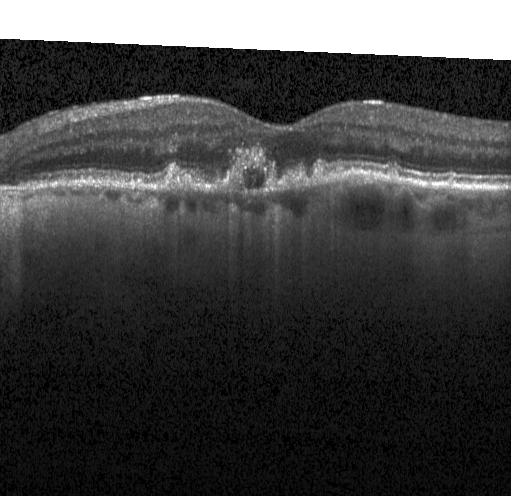 Optical coherence tomography B-scan · SD-OCT · centered on the fovea — Finding: choroidal neovascularization (CNV).